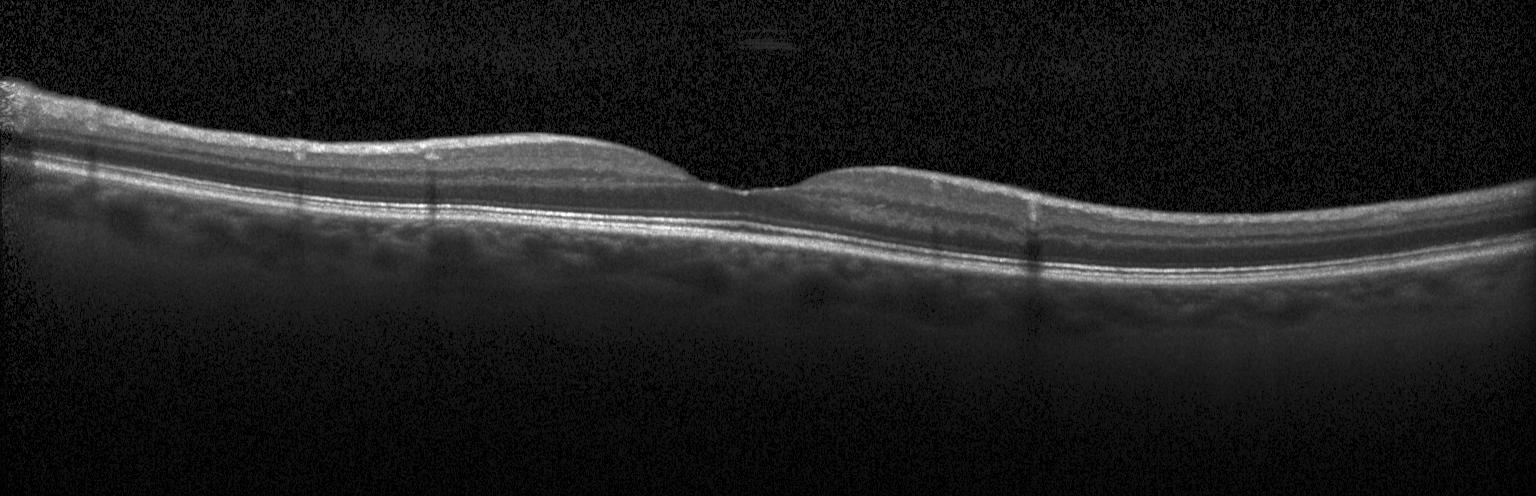

Retinal OCT cross-section showing no choroidal neovascularization, no diabetic macular edema, and no drusen.